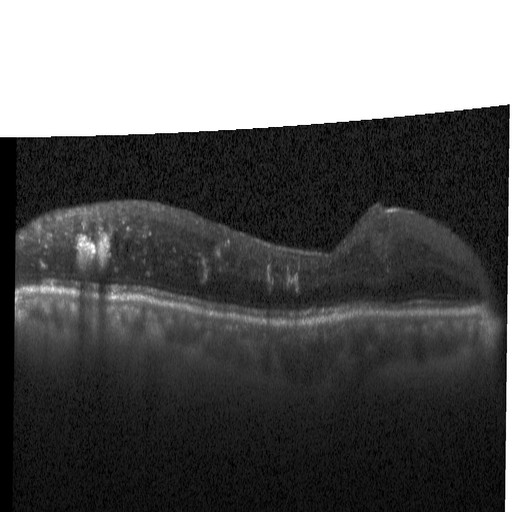
Retinal OCT cross-section.
The scan shows DME.